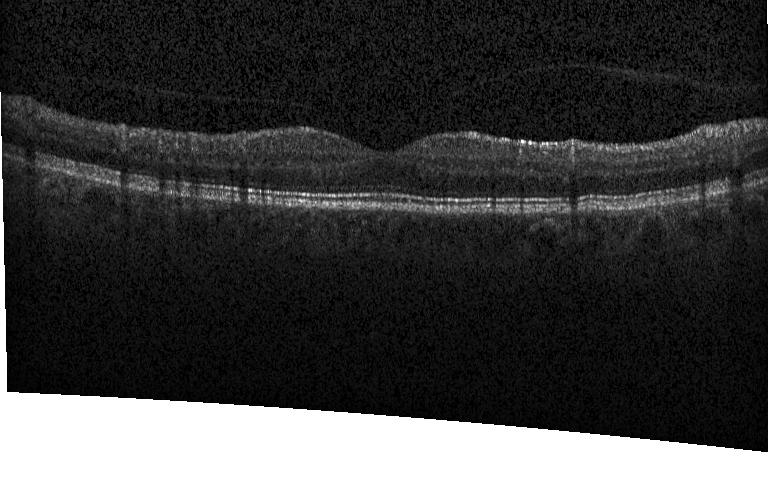 Macular scan, OCT B-scan — Impression: no evidence of choroidal neovascularization, diabetic macular edema, or drusen.